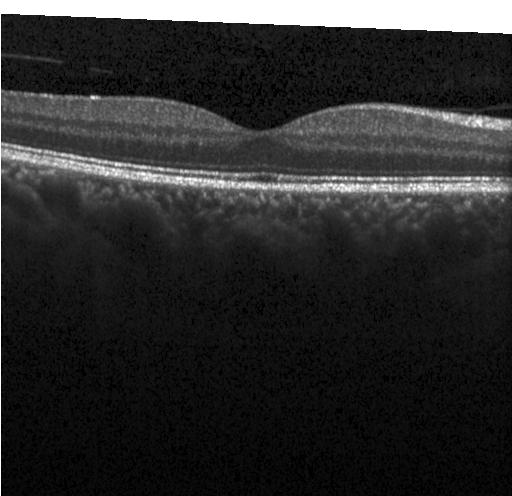

Fovea-centered · OCT B-scan · spectral-domain optical coherence tomography. Assessment: neither choroidal neovascularization, diabetic macular edema, nor drusen.